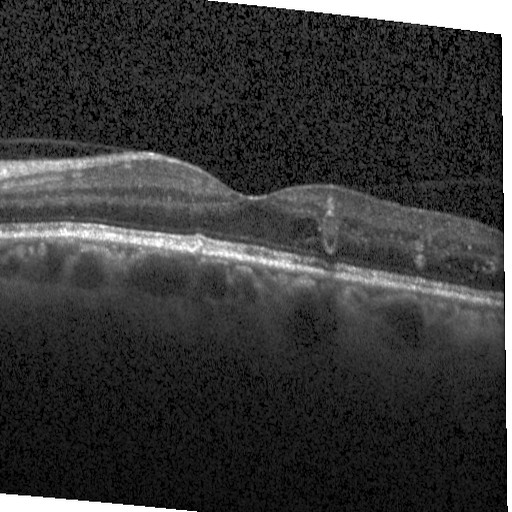
Through the macula, spectral-domain OCT, optical coherence tomography scan.
Macular OCT: DME.